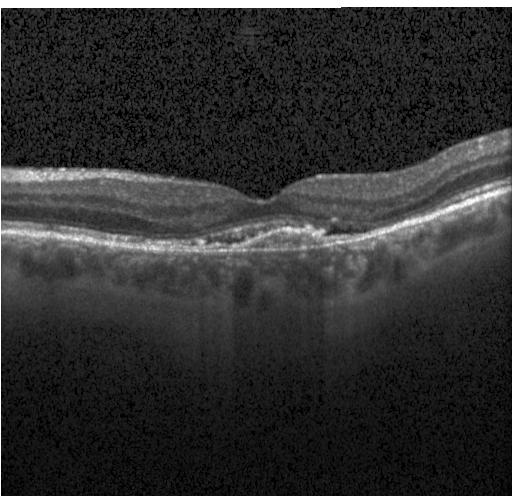
Impression: a choroidal neovascular membrane.